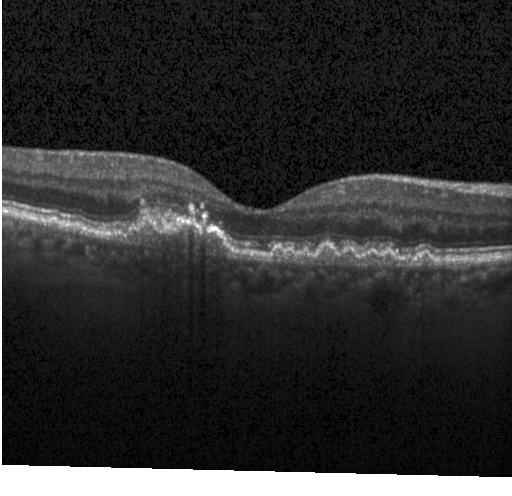 Optical coherence tomography scan.
Finding: choroidal neovascularization.